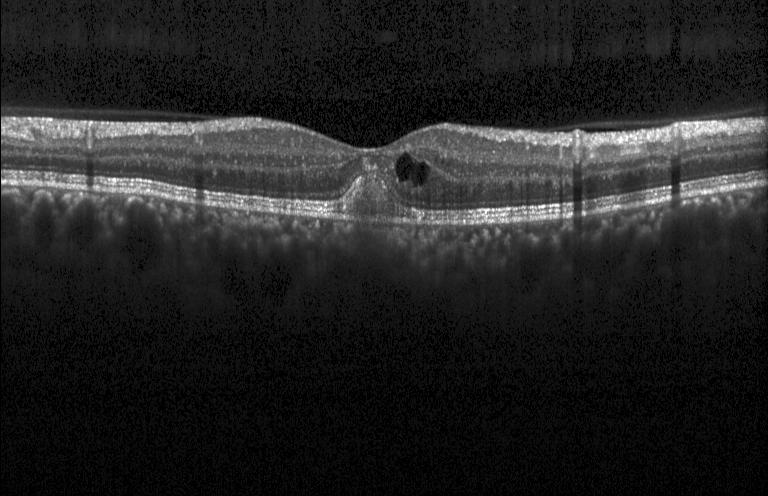 SD-OCT; Heidelberg Spectralis OCT system; OCT line scan; macular scan. The scan shows choroidal neovascularization (CNV).